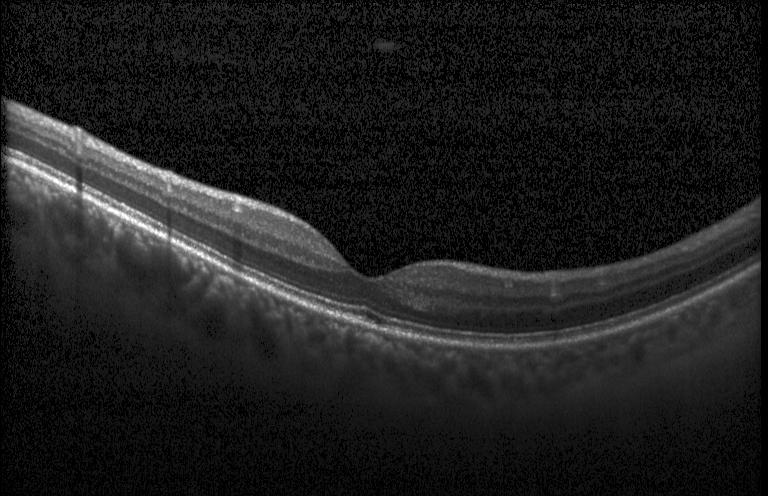

Diagnosis: no CNV, no DME, and no drusen.